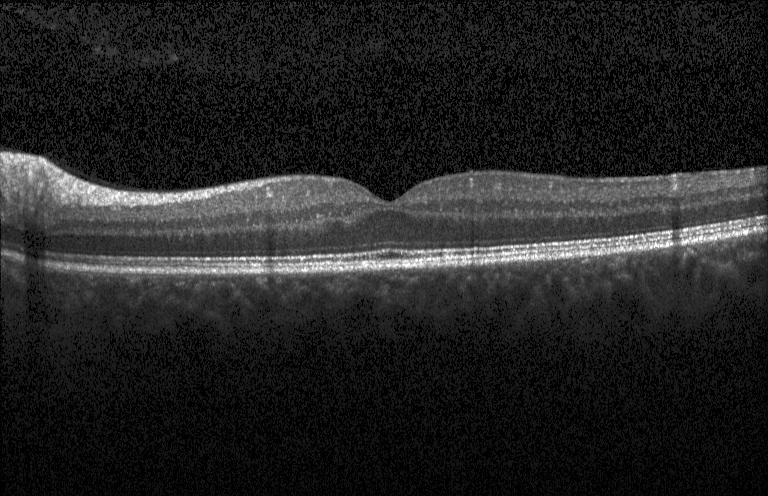

Macular OCT: neither choroidal neovascularization, diabetic macular edema, nor drusen.